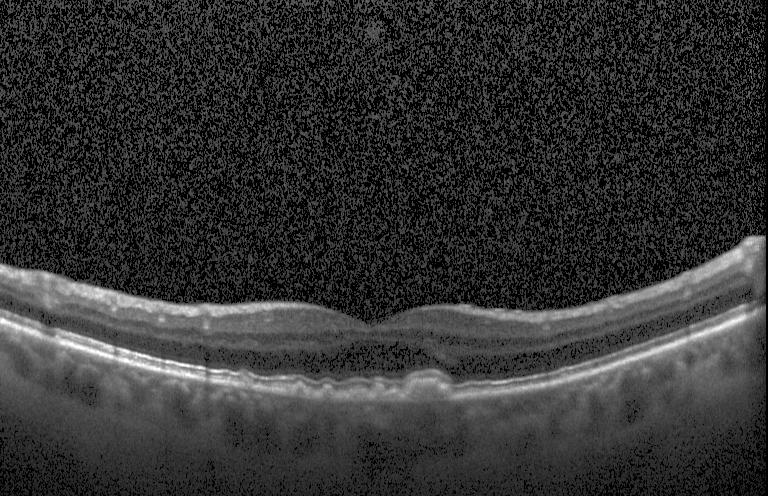 OCT finding: sub-RPE drusenoid deposits.